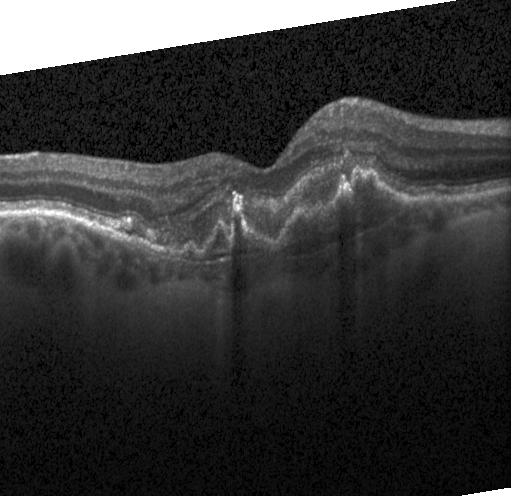
Macular OCT demonstrating a choroidal neovascular membrane.